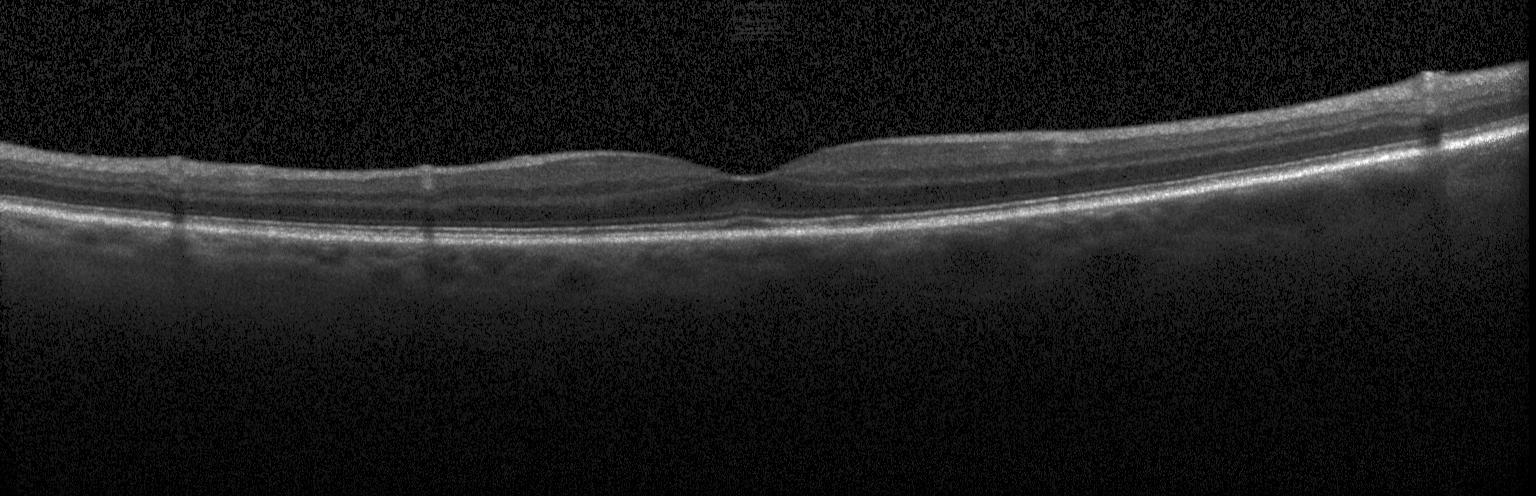

Optical coherence tomography B-scan. Diagnosis: no choroidal neovascularization, no diabetic macular edema, and no drusen.